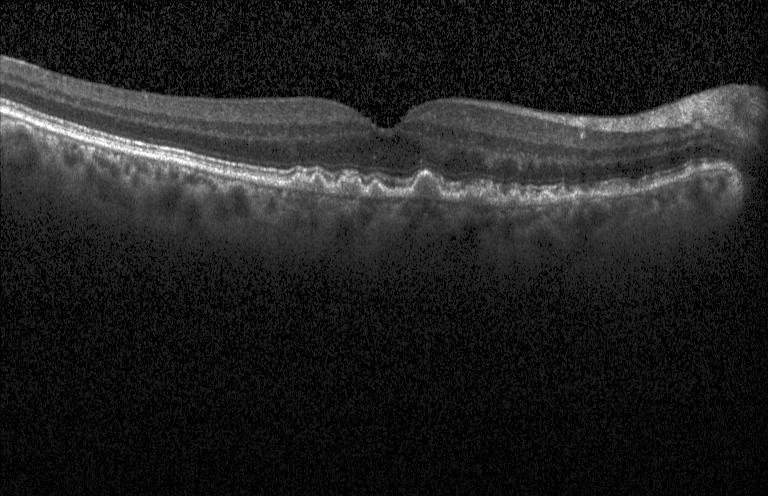 Retinal OCT cross-section; SD-OCT
Assessment: sub-RPE drusenoid deposits.